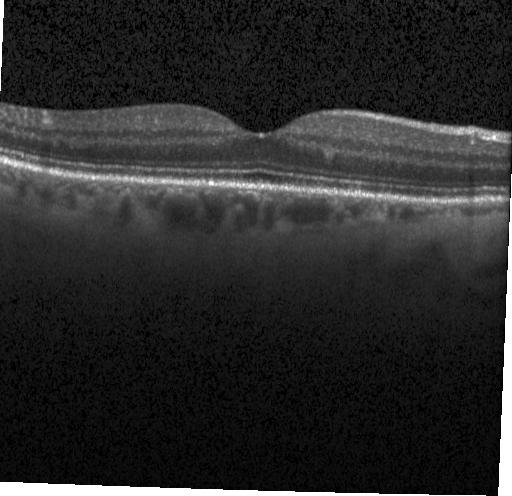 Instrument: Heidelberg Spectralis · retinal OCT cross-section · centered on the fovea
Impression: neither CNV, DME, nor drusen.